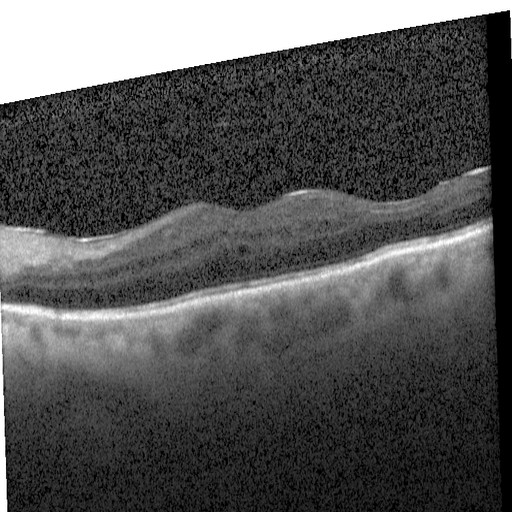

OCT B-scan showing diabetic macular edema (DME).